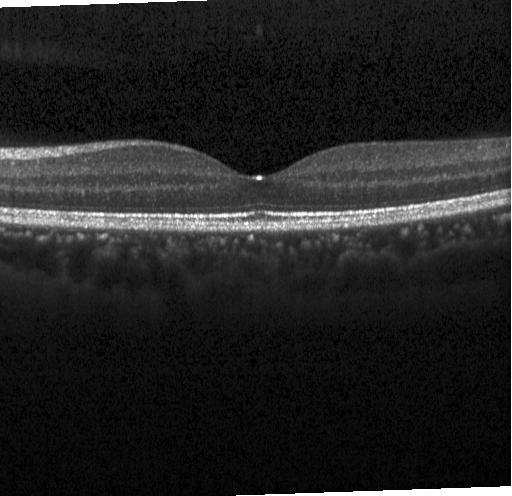
Optical coherence tomography B-scan. Instrument: Heidelberg Spectralis.
Finding: neither CNV, DME, nor drusen.